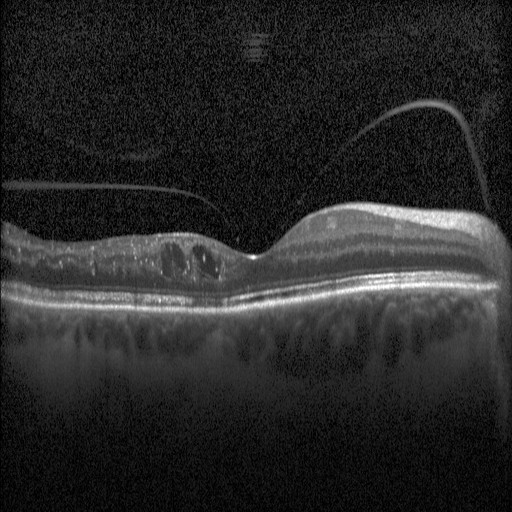

Retinal OCT cross-section showing diabetic macular edema (DME).